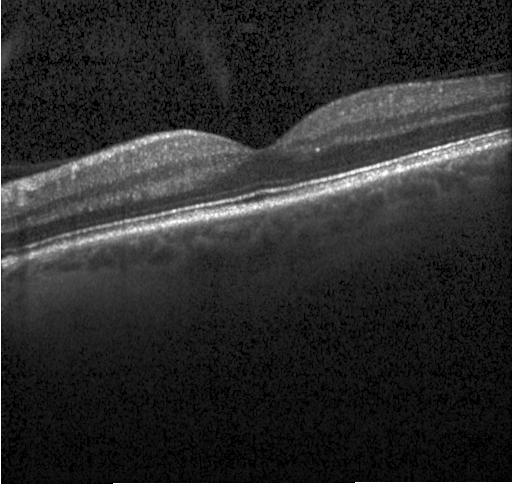
Diagnosis: no choroidal neovascularization, no diabetic macular edema, and no drusen.